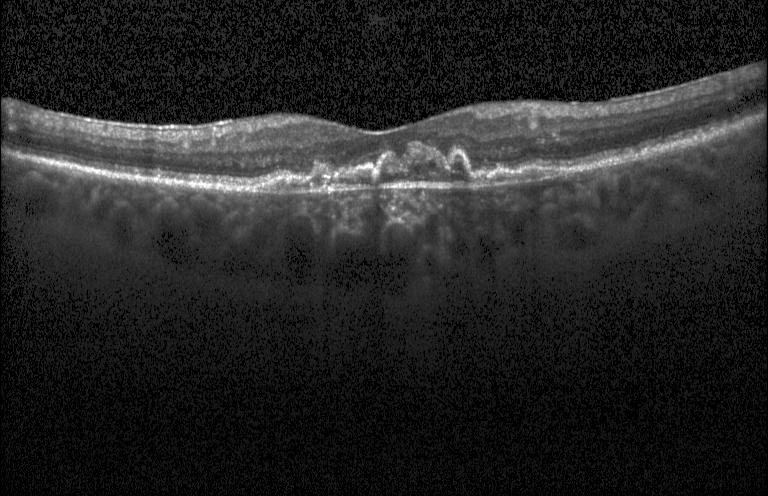
This B-scan demonstrates choroidal neovascularization (CNV).